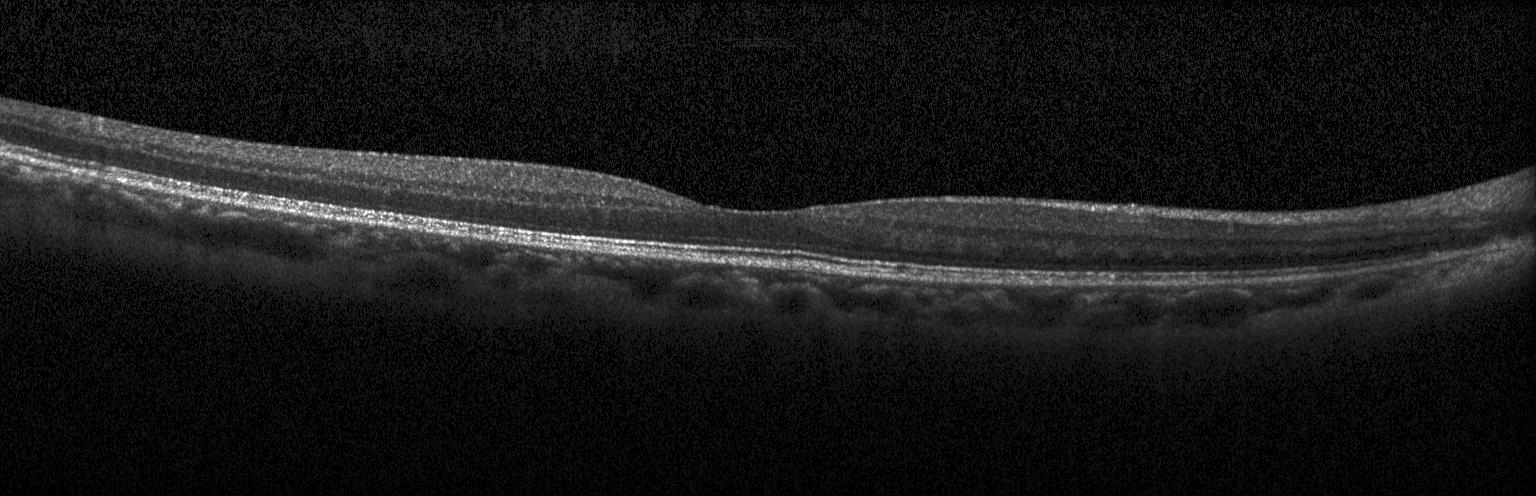 Spectral-domain OCT B-scan: no choroidal neovascularization, diabetic macular edema, or drusen.